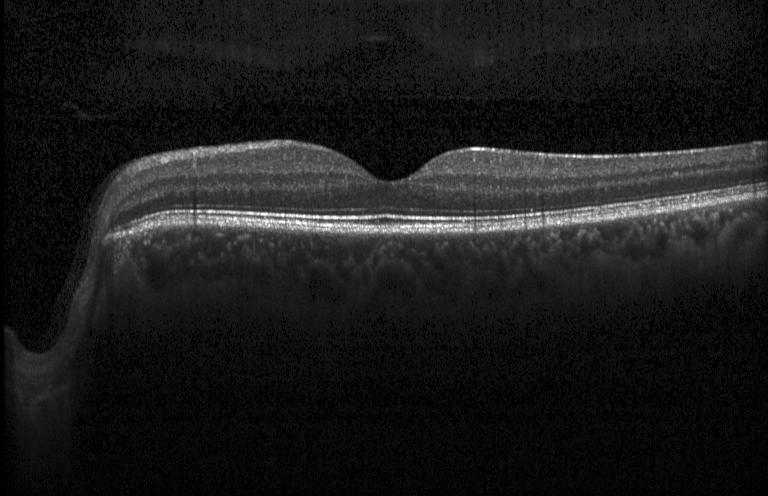
SD-OCT. Heidelberg Spectralis. OCT line scan. Through the macula.
Neither CNV, DME, nor drusen.